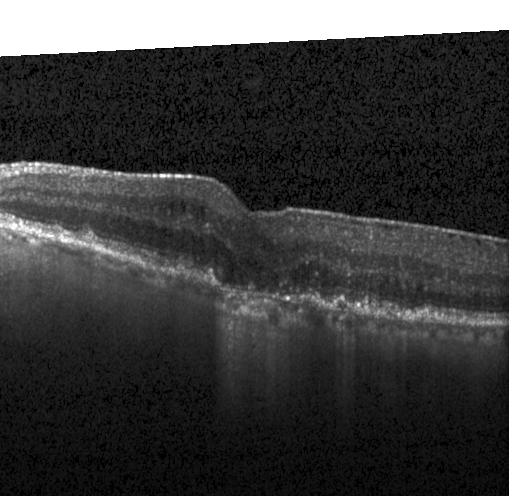
Spectral-domain optical coherence tomography, macular scan, optical coherence tomography scan — OCT finding: a choroidal neovascular membrane.